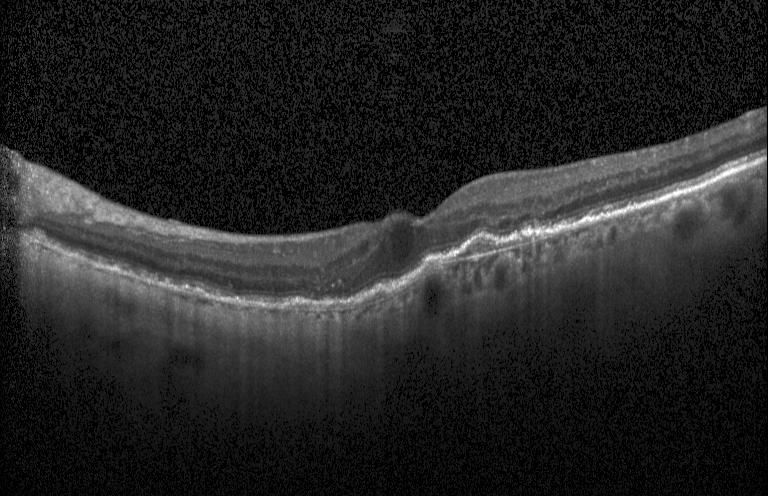 Dx: a choroidal neovascular membrane.